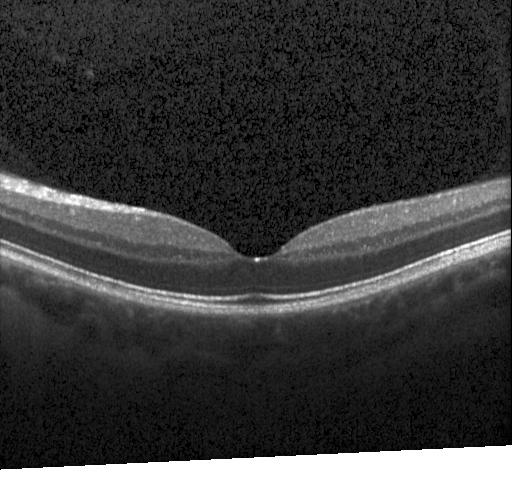

Optical coherence tomography B-scan · Heidelberg Spectralis OCT system.
The scan shows neither CNV, DME, nor drusen.